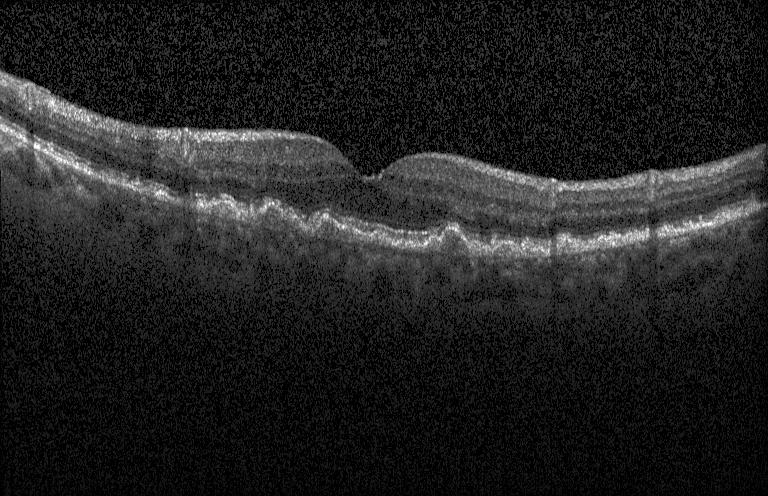

OCT line scan. Finding: multiple drusen.